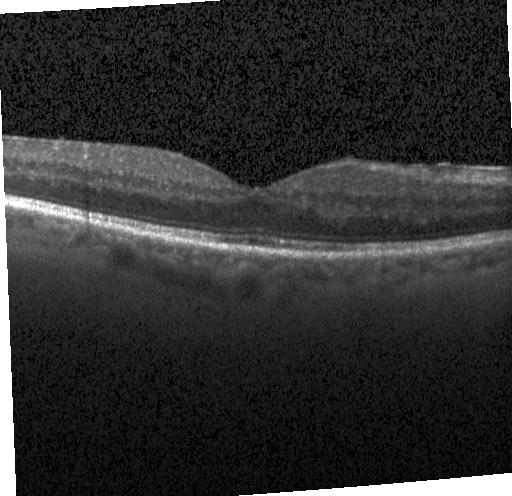

OCT line scan — Finding: no evidence of CNV, DME, or drusen.